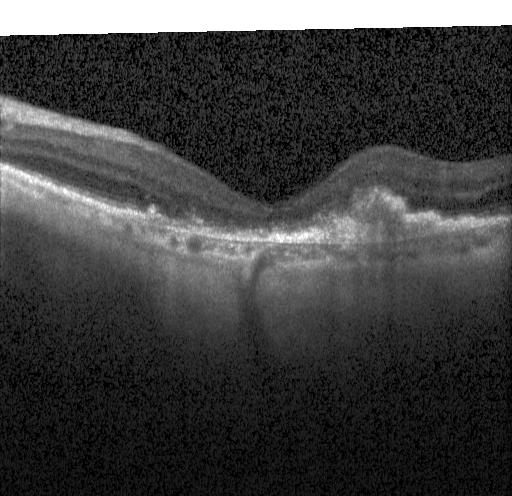 Finding: choroidal neovascularization (CNV).